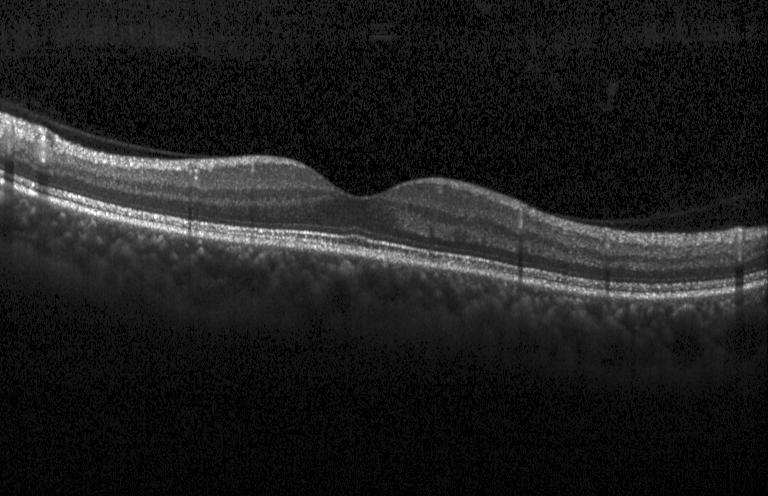
Heidelberg Spectralis OCT system · SD-OCT · optical coherence tomography B-scan
Impression: no CNV, no DME, and no drusen.